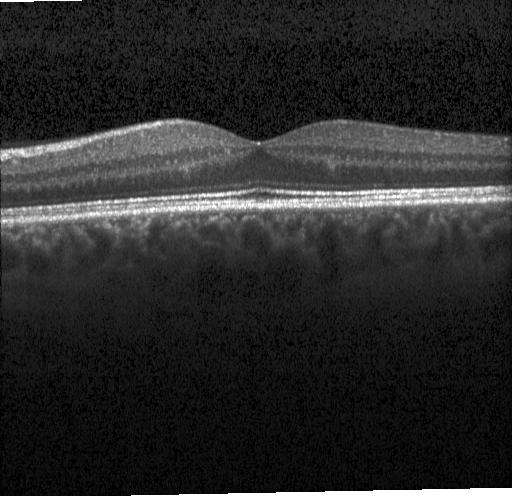 SD-OCT. Through the macula. OCT line scan. Heidelberg Spectralis OCT system — This B-scan demonstrates no choroidal neovascularization, no diabetic macular edema, and no drusen.